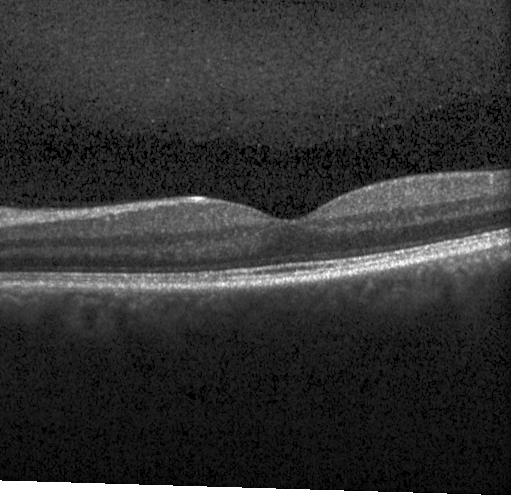

SD-OCT; OCT B-scan.
Diagnosis: no evidence of CNV, DME, or drusen.